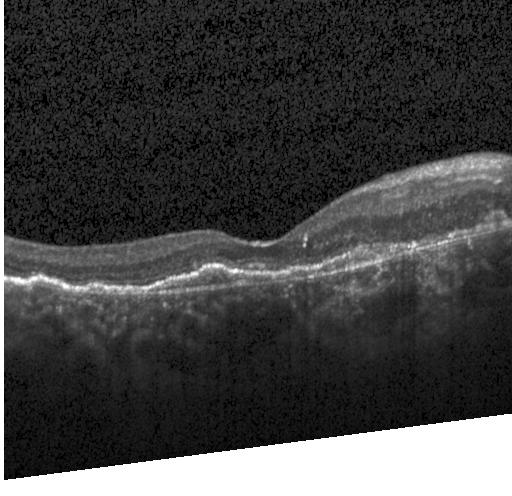

Spectral-domain OCT; macular scan; retinal OCT cross-section
OCT finding: CNV.